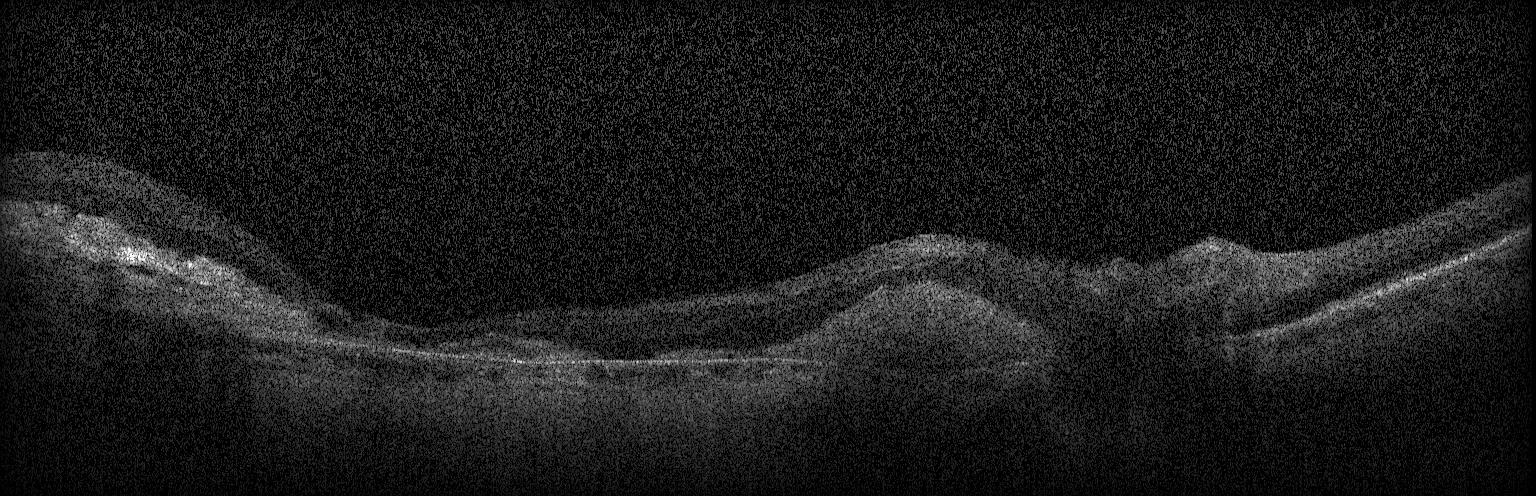
Impression: CNV.